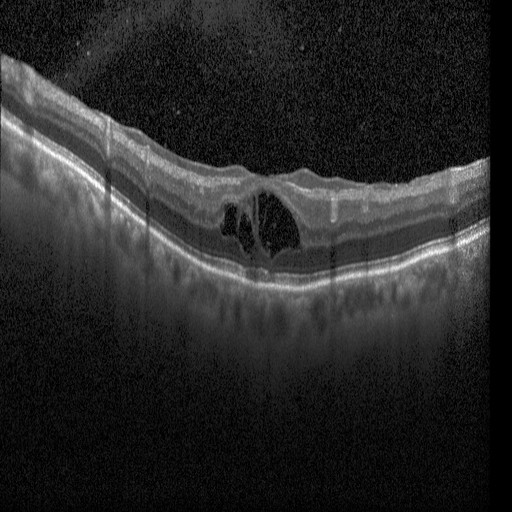
Optical coherence tomography B-scan. Through the macula — Impression: DME.